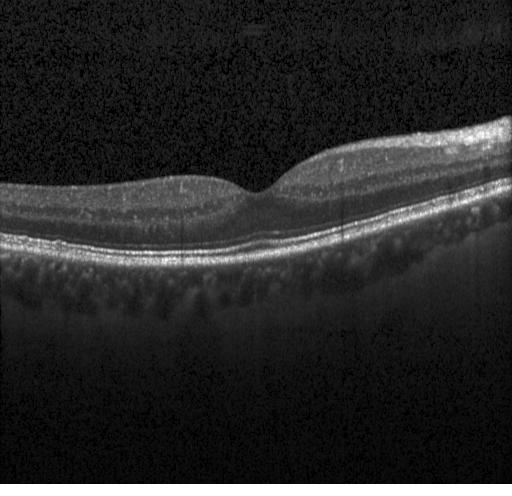 Spectral-domain optical coherence tomography. OCT line scan
The scan shows no evidence of choroidal neovascularization, diabetic macular edema, or drusen.